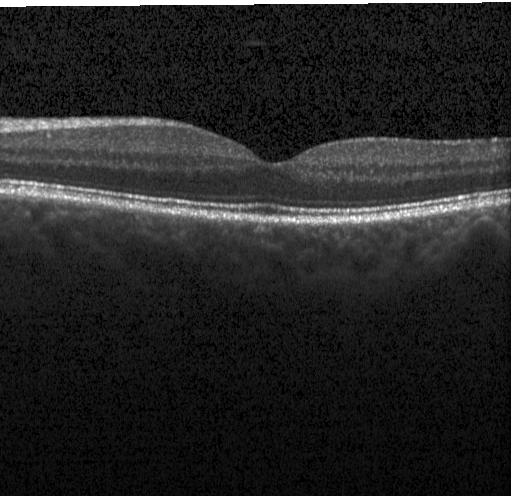

Finding: no evidence of choroidal neovascularization, diabetic macular edema, or drusen.